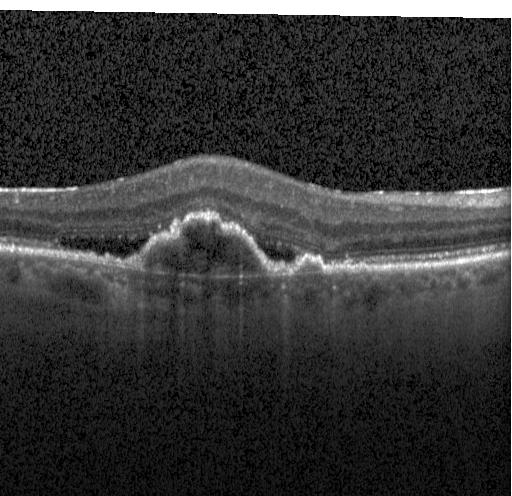

Spectral-domain optical coherence tomography, acquired on a Heidelberg Spectralis, through the macula, OCT B-scan — Assessment: a choroidal neovascular membrane.